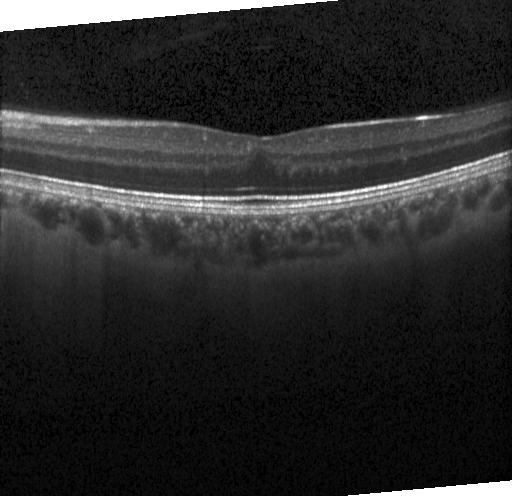
Spectral-domain OCT B-scan: no choroidal neovascularization, diabetic macular edema, or drusen.